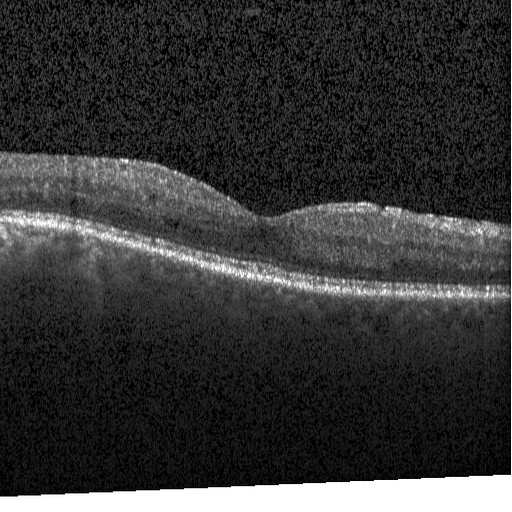

Macular OCT demonstrating diabetic macular edema (DME).